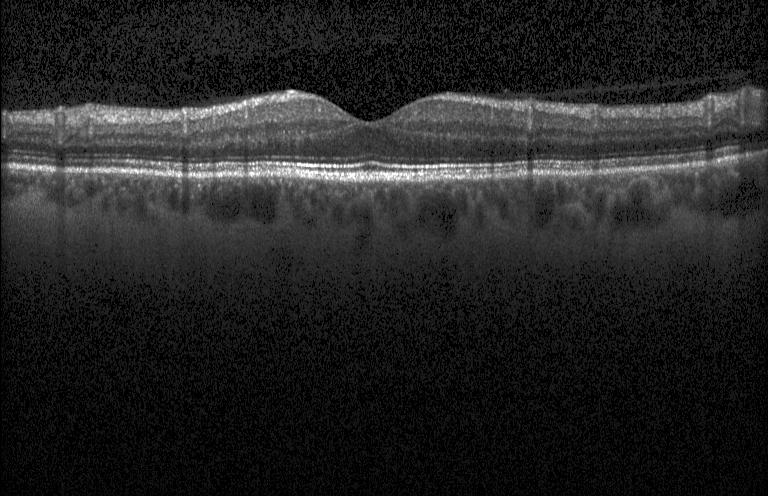
Optical coherence tomography scan. Diagnosis: no evidence of CNV, DME, or drusen.